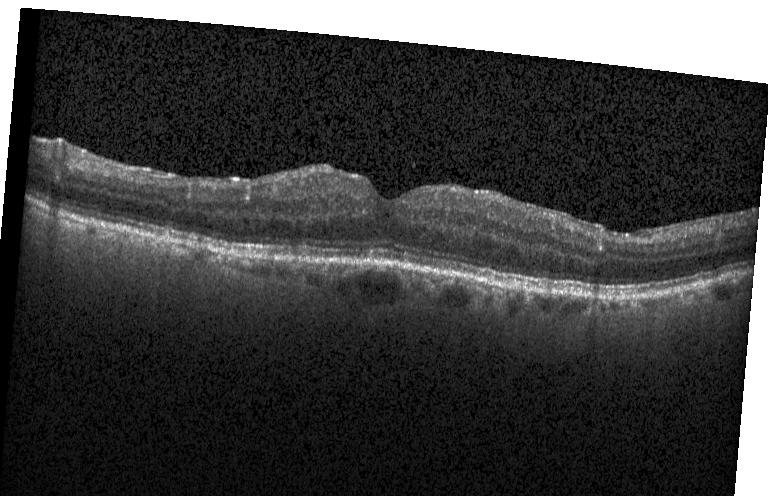

Optical coherence tomography scan — The scan shows no choroidal neovascularization, diabetic macular edema, or drusen.